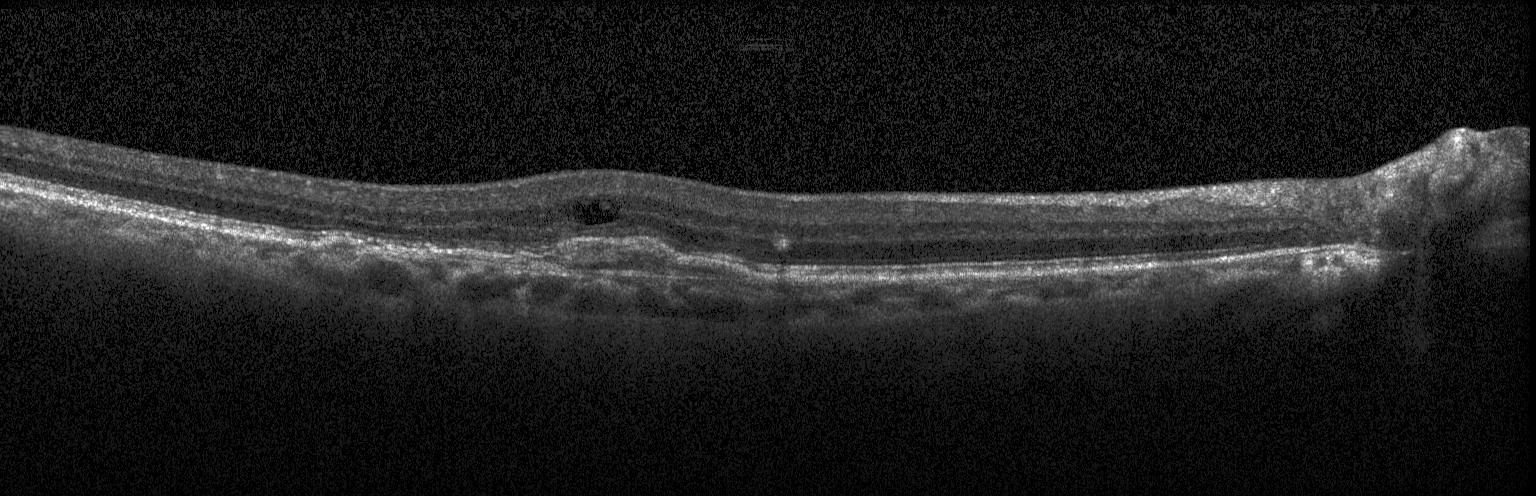 Macular scan; retinal OCT cross-section; spectral-domain OCT; Heidelberg Spectralis. CNV.